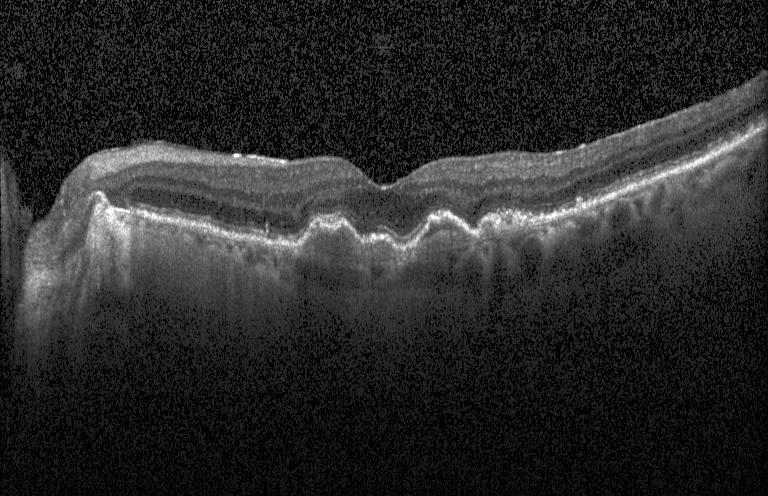
Optical coherence tomography B-scan — Impression: a choroidal neovascular membrane.